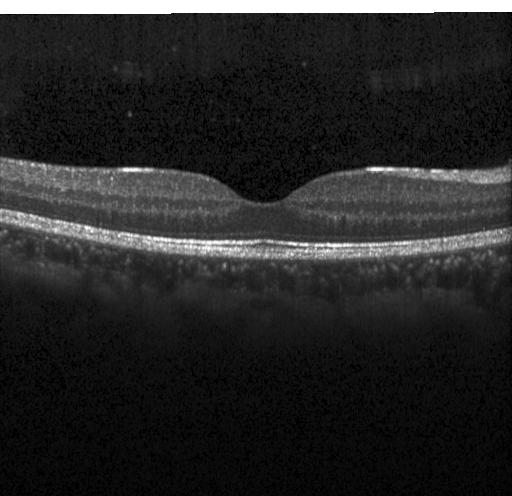 No choroidal neovascularization, diabetic macular edema, or drusen.